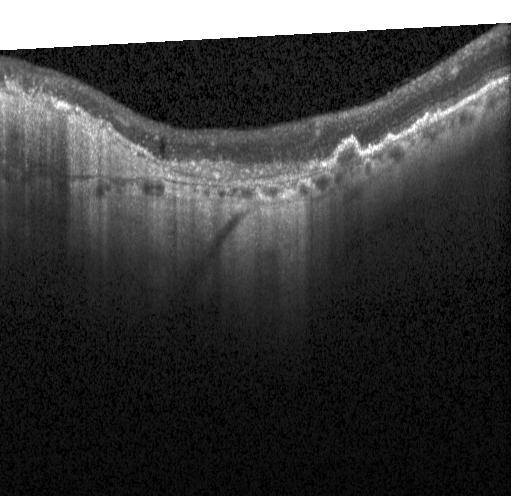 Fovea-centered · OCT line scan · Heidelberg Spectralis OCT system
Dx: a choroidal neovascular membrane.